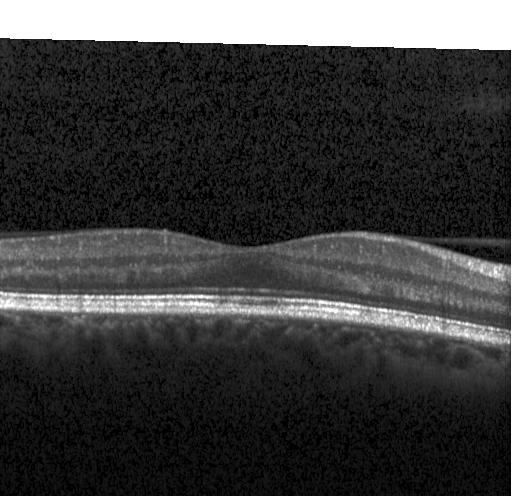
Retinal OCT B-scan.
Neither choroidal neovascularization, diabetic macular edema, nor drusen.